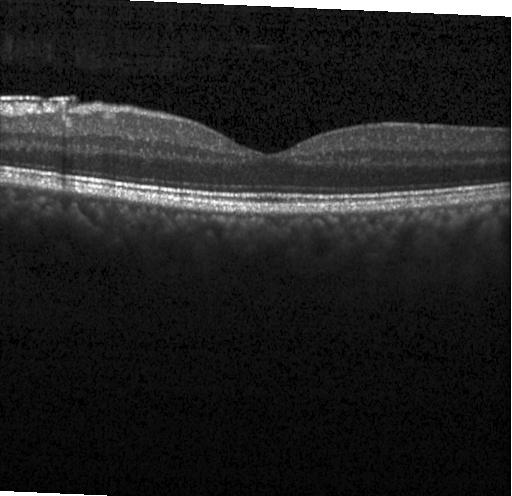 OCT B-scan · spectral-domain OCT · fovea-centered · Heidelberg Spectralis OCT system.
The scan shows neither CNV, DME, nor drusen.